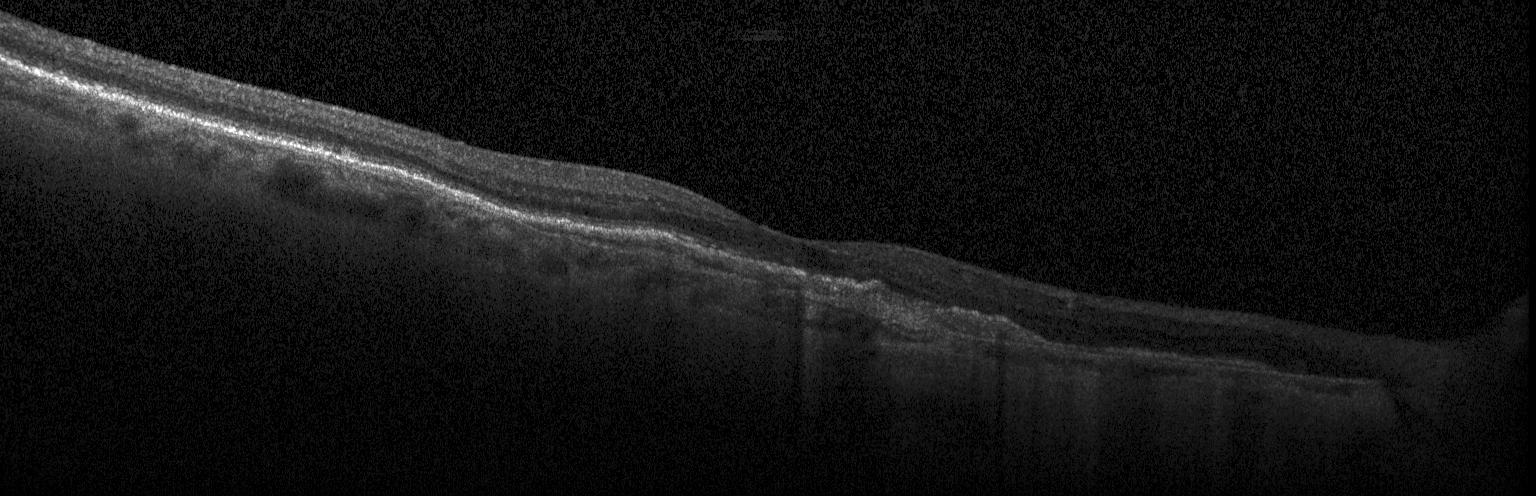
Dx: choroidal neovascularization (CNV).